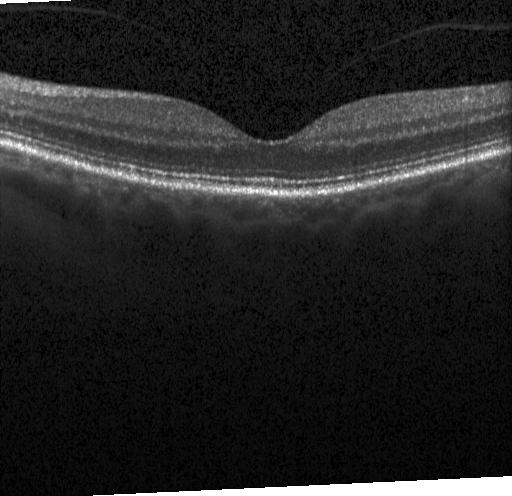
Spectral-domain optical coherence tomography · macular scan · OCT line scan
This B-scan demonstrates no choroidal neovascularization, no diabetic macular edema, and no drusen.